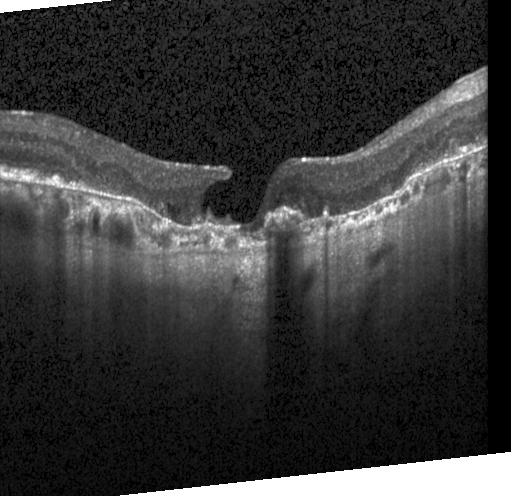

Optical coherence tomography B-scan; Heidelberg Spectralis OCT system; spectral-domain optical coherence tomography.
Impression: a choroidal neovascular membrane.